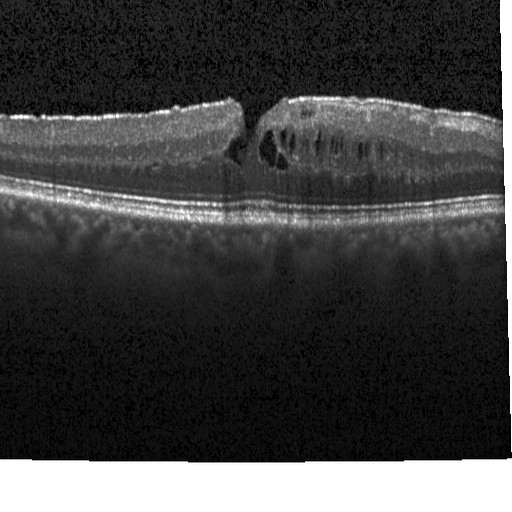

Impression: diabetic macular edema (DME).